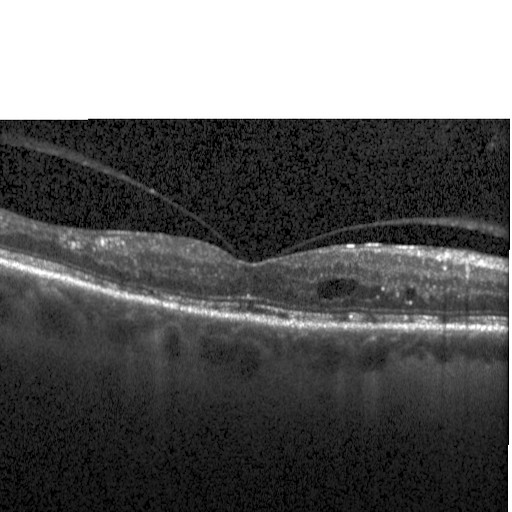

Finding: diabetic macular edema.